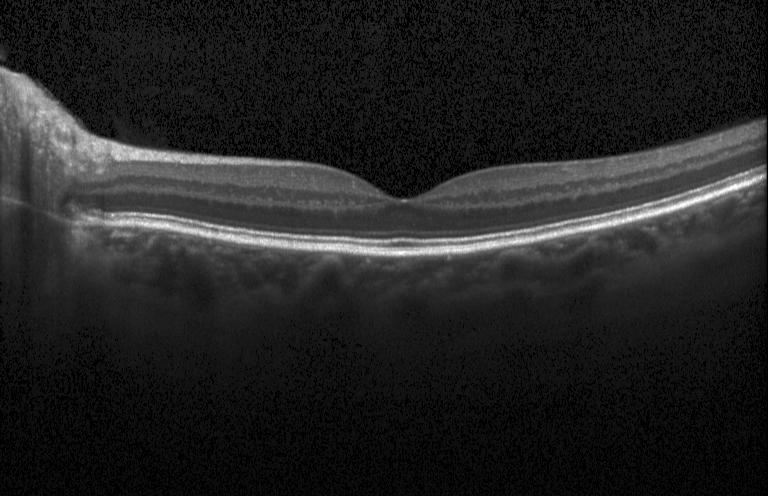

Retinal OCT B-scan, centered on the fovea, Heidelberg Spectralis OCT system — Diagnosis: neither choroidal neovascularization, diabetic macular edema, nor drusen.